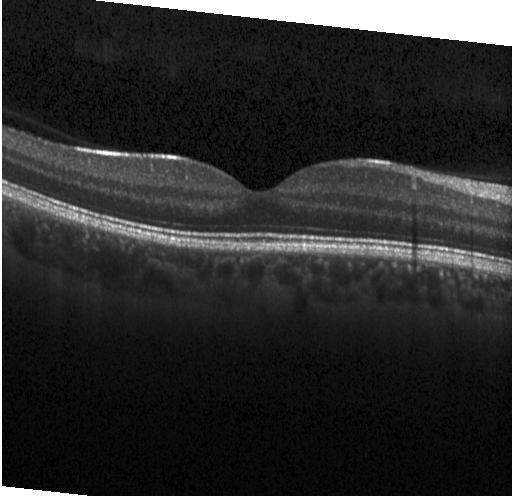

OCT B-scan showing no CNV, no DME, and no drusen.